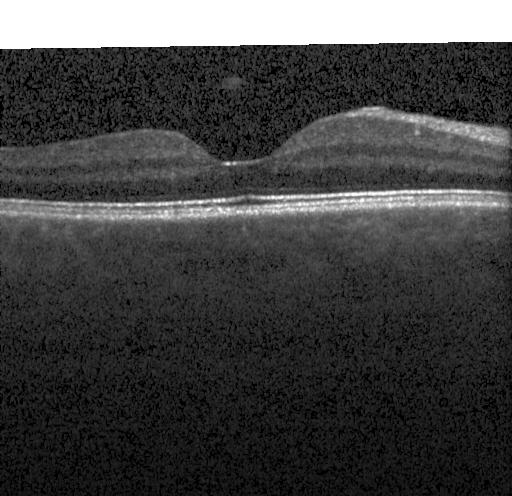 Retinal OCT B-scan; SD-OCT
The scan shows no evidence of CNV, DME, or drusen.